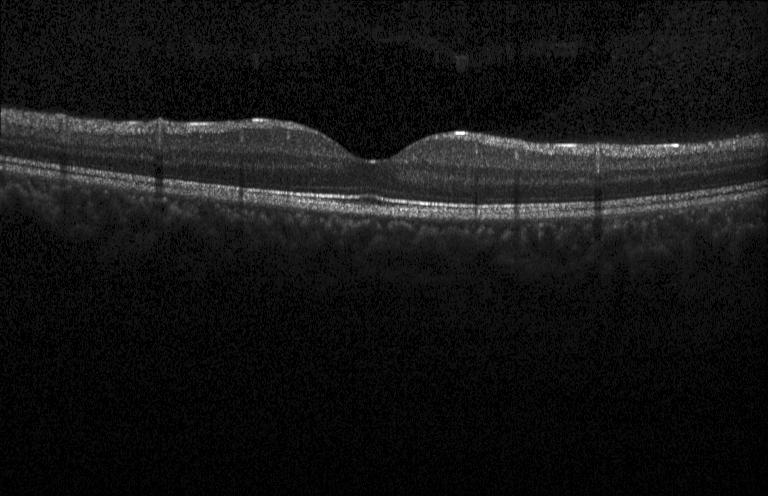

No evidence of choroidal neovascularization, diabetic macular edema, or drusen.